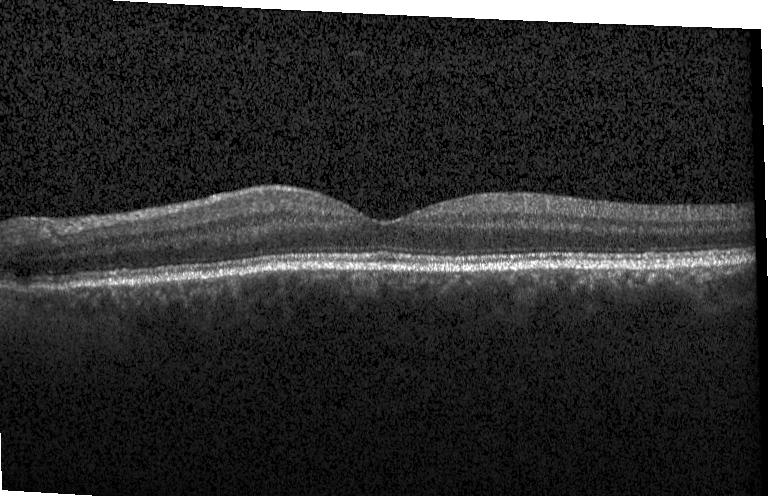
OCT B-scan
Impression: no CNV, DME, or drusen.